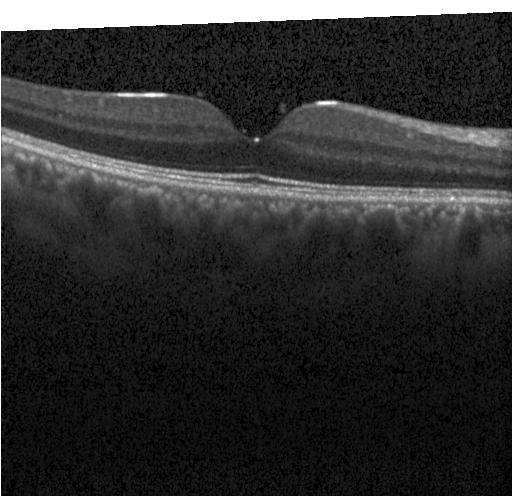
Finding: neither choroidal neovascularization, diabetic macular edema, nor drusen.